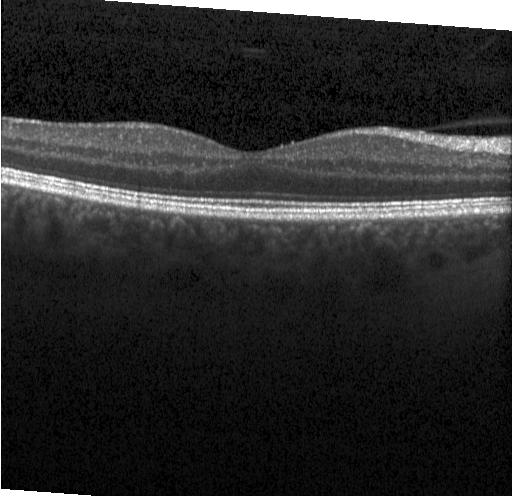

Macular OCT: neither CNV, DME, nor drusen.